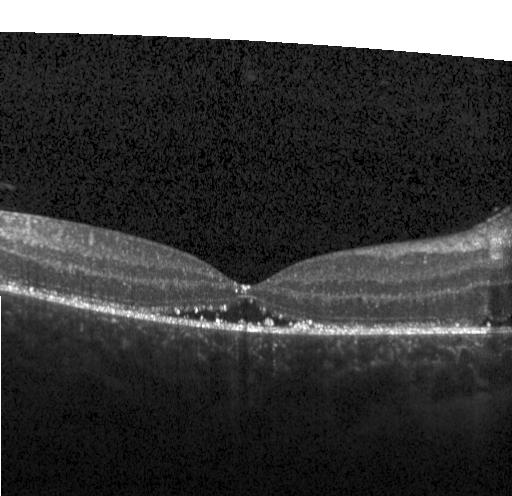
Impression: a choroidal neovascular membrane.